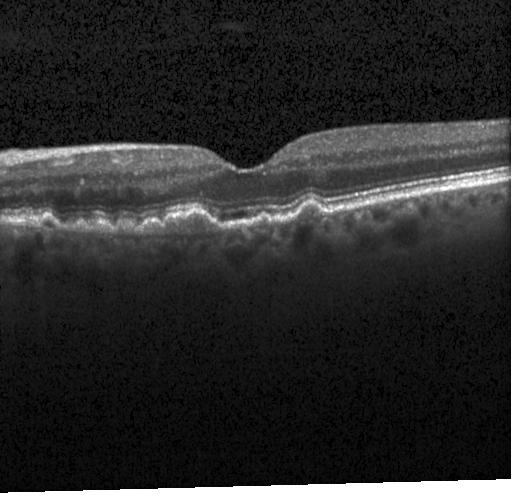
Retinal OCT B-scan. Diagnosis: drusen.